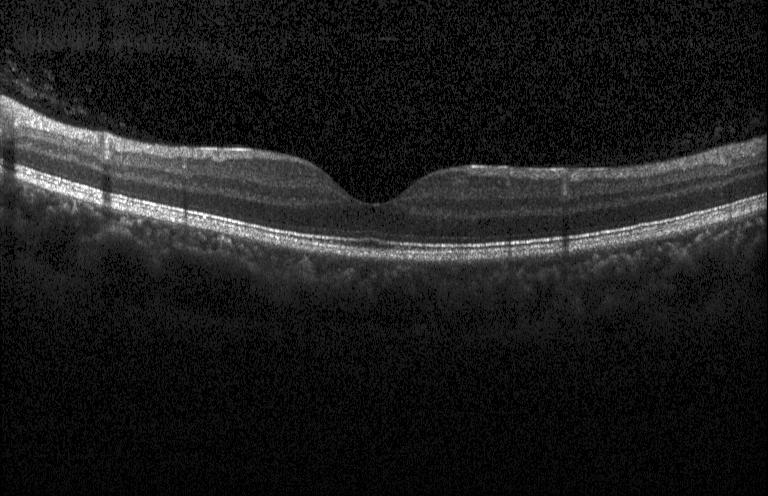
Retinal OCT B-scan · acquired on a Heidelberg Spectralis · SD-OCT.
Impression: no CNV, no DME, and no drusen.